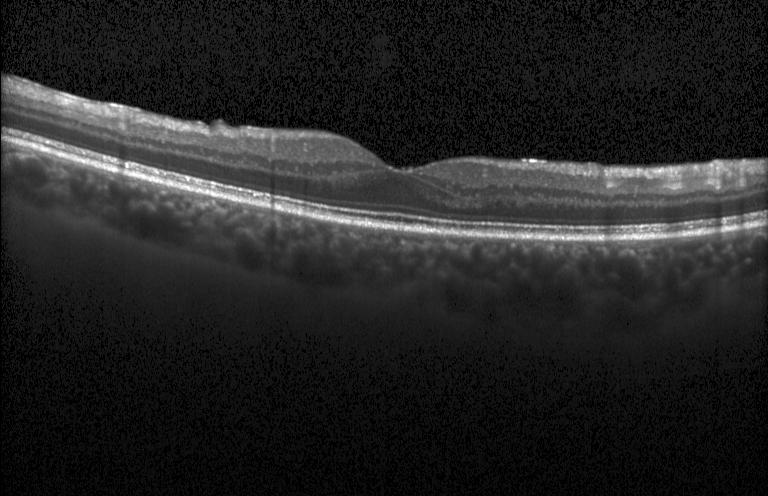
Optical coherence tomography B-scan.
This B-scan demonstrates neither choroidal neovascularization, diabetic macular edema, nor drusen.